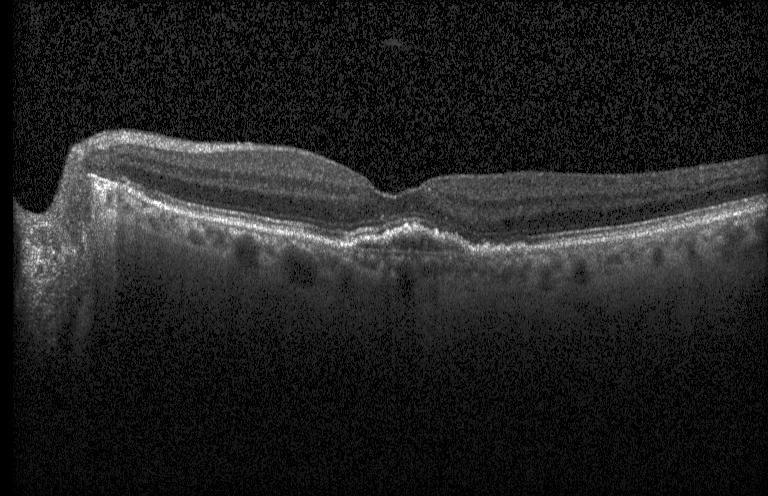

OCT line scan; fovea-centered
Finding: a choroidal neovascular membrane.